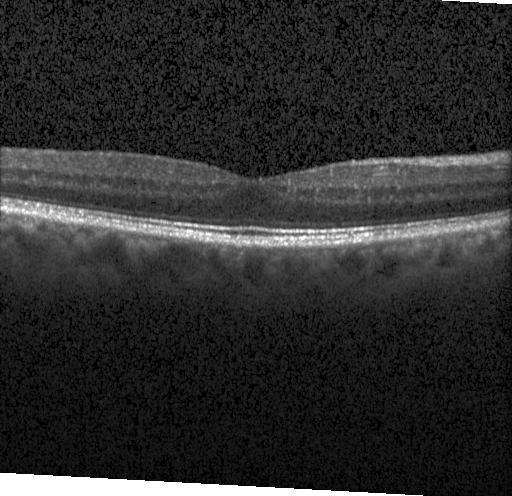

Optical coherence tomography B-scan.
Diagnosis: no CNV, no DME, and no drusen.